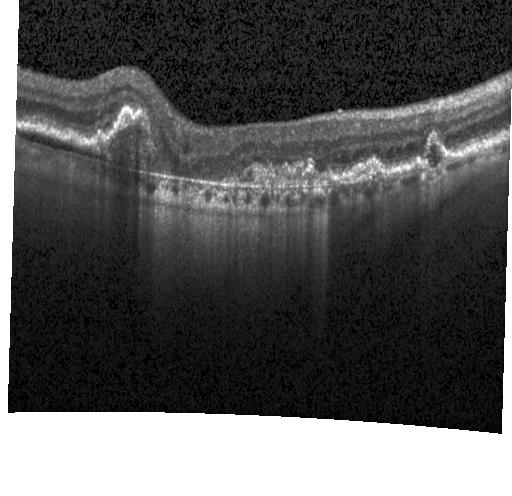 OCT line scan. Instrument: Heidelberg Spectralis. Spectral-domain OCT. Horizontal scan through the fovea. Macular OCT: a choroidal neovascular membrane.